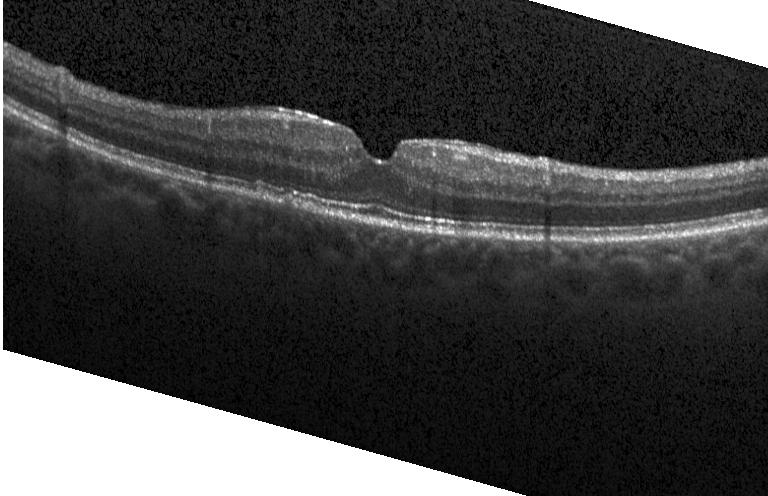
OCT B-scan. Diagnosis: sub-RPE drusenoid deposits.